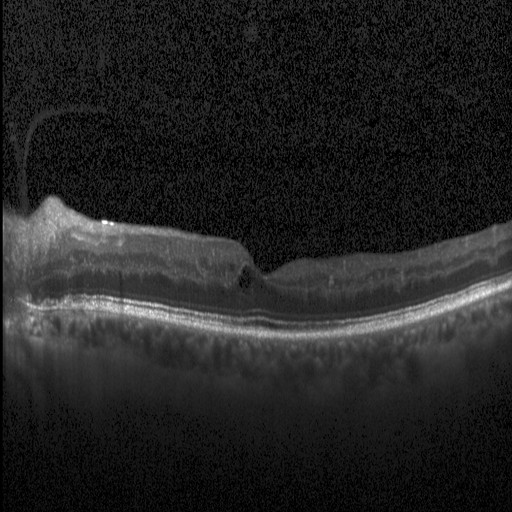 Centered on the fovea, retinal OCT cross-section, instrument: Heidelberg Spectralis — Assessment: DME.